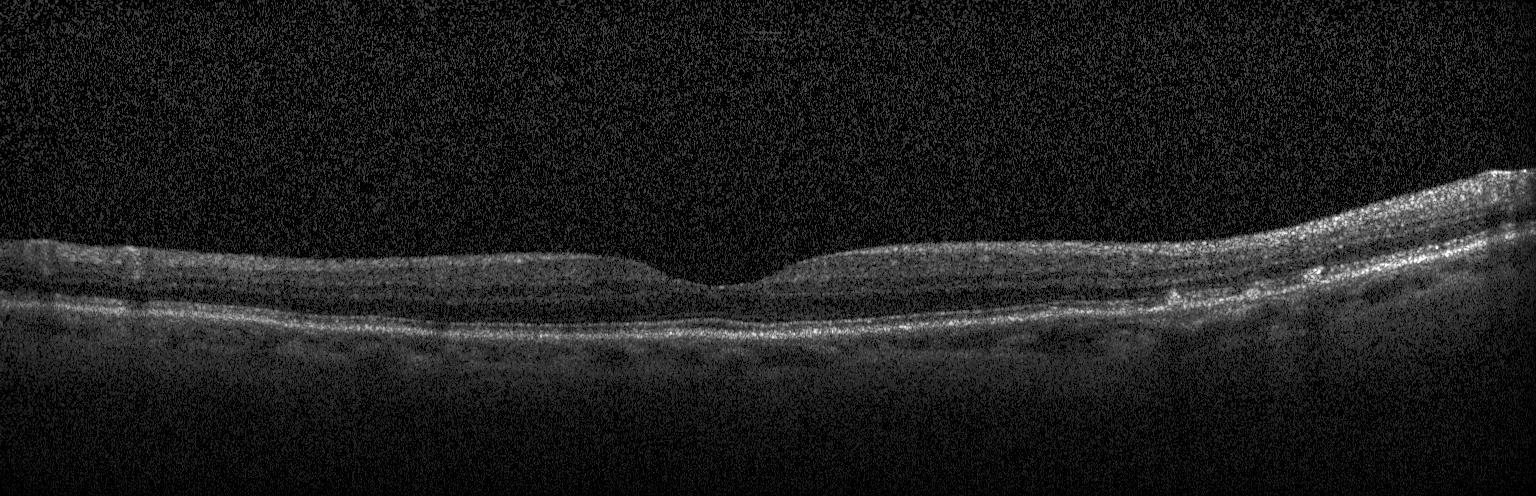 OCT B-scan — Impression: drusen.